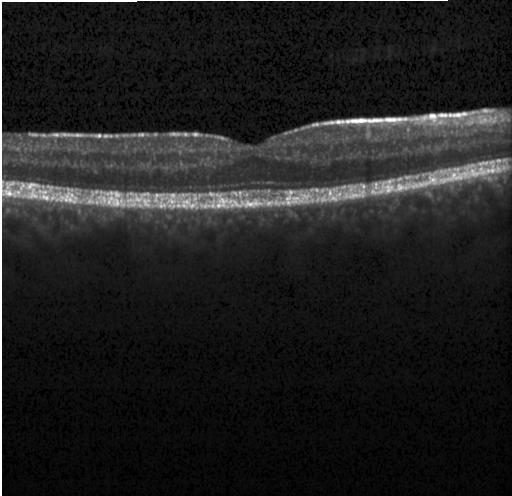
Spectral-domain OCT. Heidelberg Spectralis. Fovea-centered. OCT line scan — Dx: no evidence of CNV, DME, or drusen.